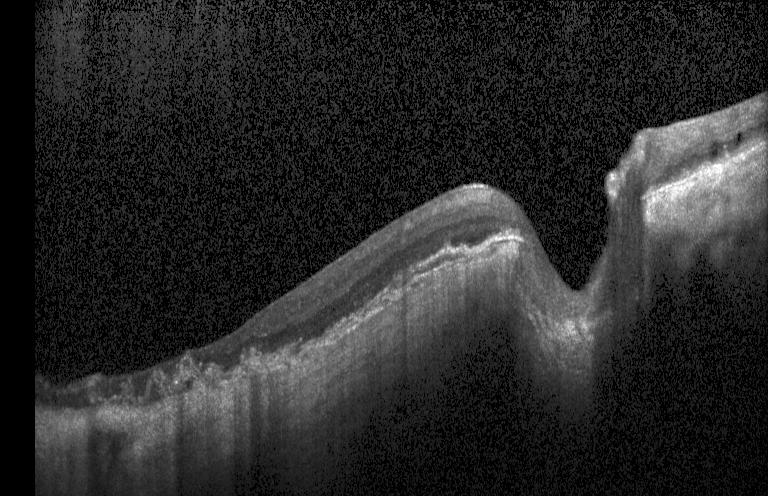
Macular OCT: a choroidal neovascular membrane.